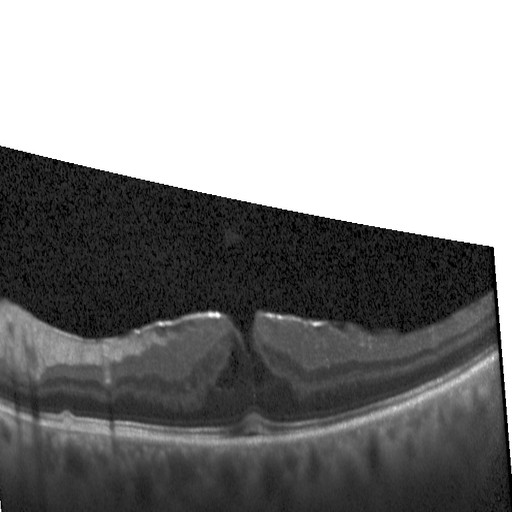
OCT finding: diabetic macular edema (DME).